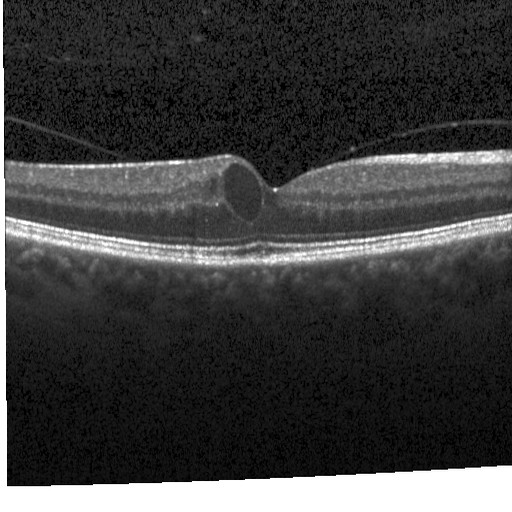 This B-scan demonstrates diabetic macular edema.